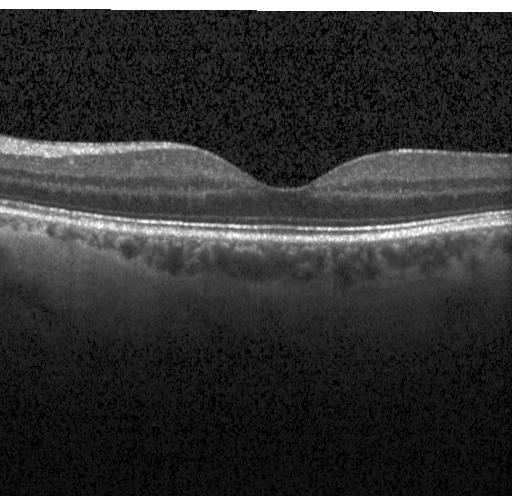

Heidelberg Spectralis OCT system · through the macula · optical coherence tomography scan. Assessment: no choroidal neovascularization, diabetic macular edema, or drusen.